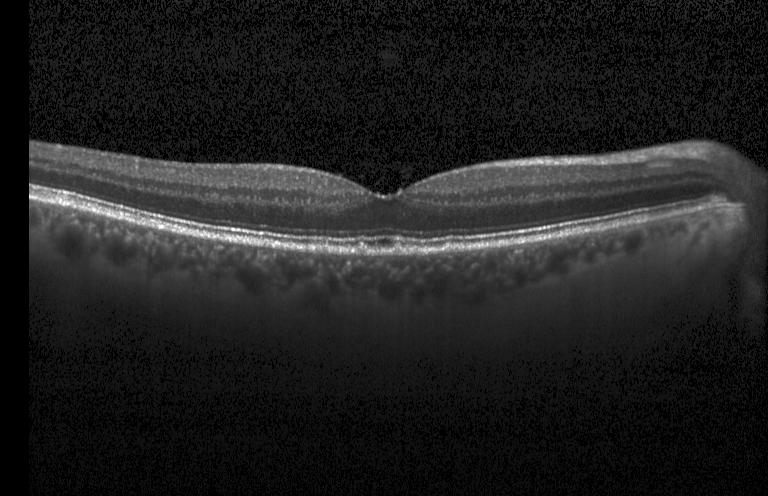

Retinal OCT cross-section showing sub-RPE drusenoid deposits.